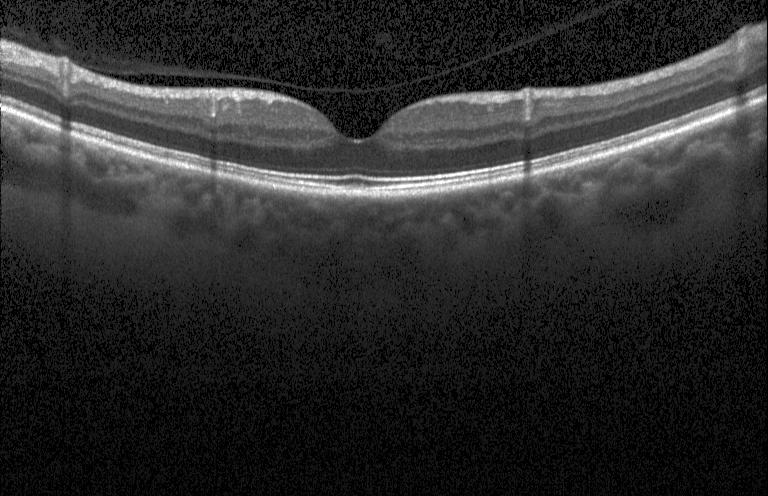

Instrument: Heidelberg Spectralis. Spectral-domain optical coherence tomography. Optical coherence tomography scan — Finding: no choroidal neovascularization, diabetic macular edema, or drusen.